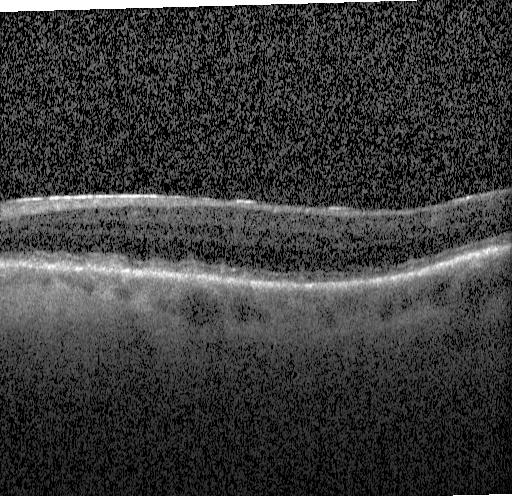
Spectral-domain OCT, Heidelberg Spectralis, OCT B-scan, horizontal scan through the fovea.
Finding: sub-RPE drusenoid deposits.